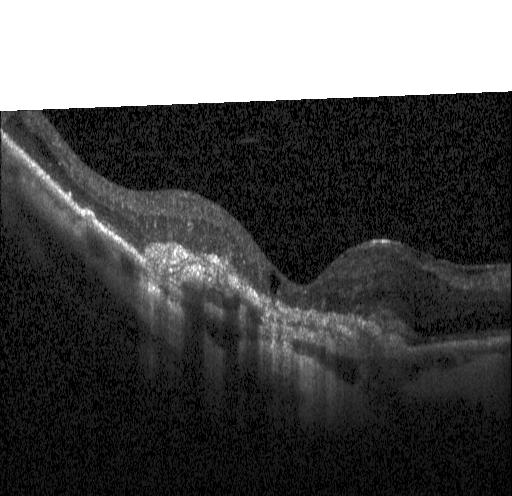

Retinal OCT B-scan — A choroidal neovascular membrane.